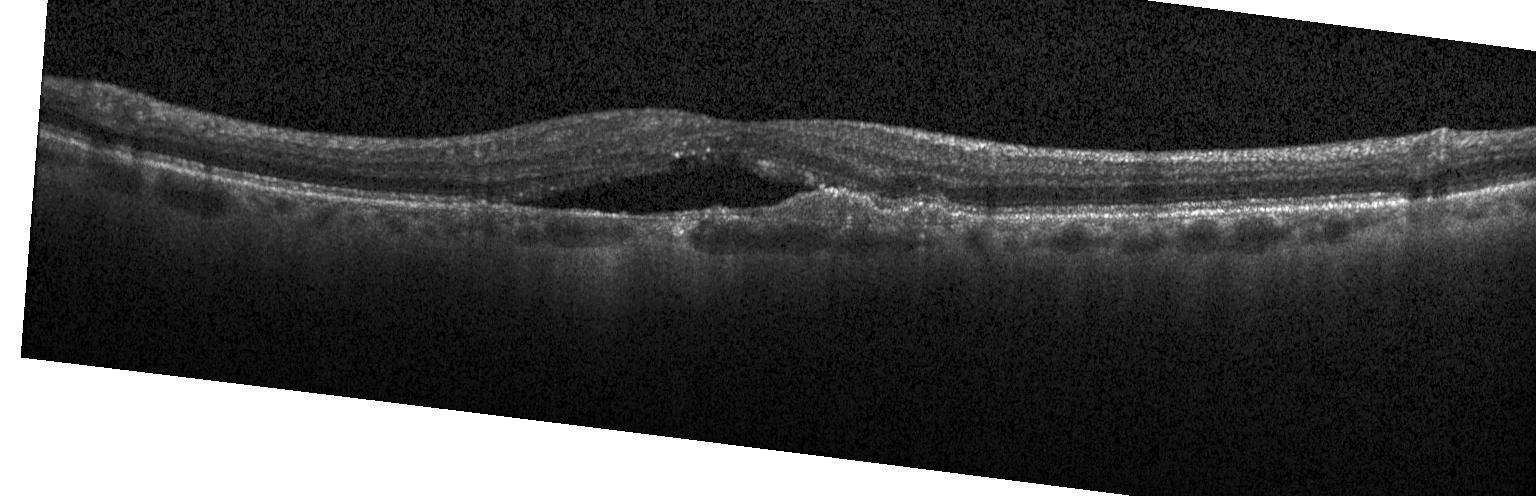

OCT B-scan showing a choroidal neovascular membrane.